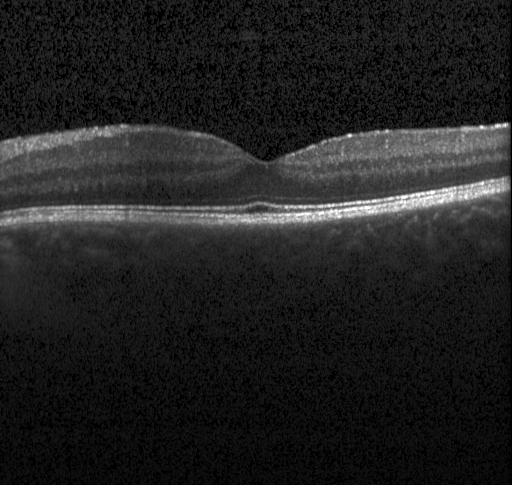
Optical coherence tomography scan · Heidelberg Spectralis OCT system · horizontal scan through the fovea · SD-OCT
No evidence of CNV, DME, or drusen.